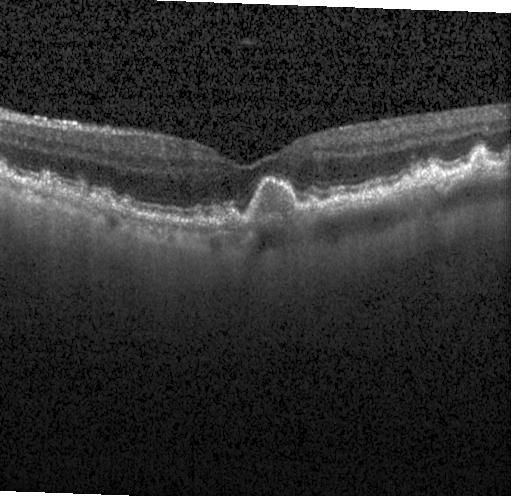

Horizontal scan through the fovea. OCT line scan. Instrument: Heidelberg Spectralis. Spectral-domain optical coherence tomography — Diagnosis: sub-RPE drusenoid deposits.